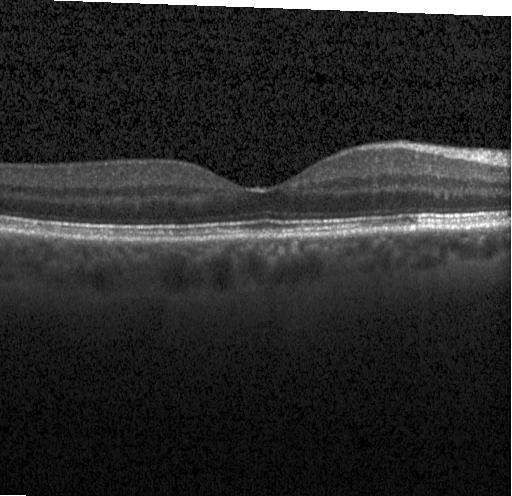 Retinal OCT cross-section; horizontal scan through the fovea; instrument: Heidelberg Spectralis; spectral-domain OCT — Diagnosis: no CNV, no DME, and no drusen.